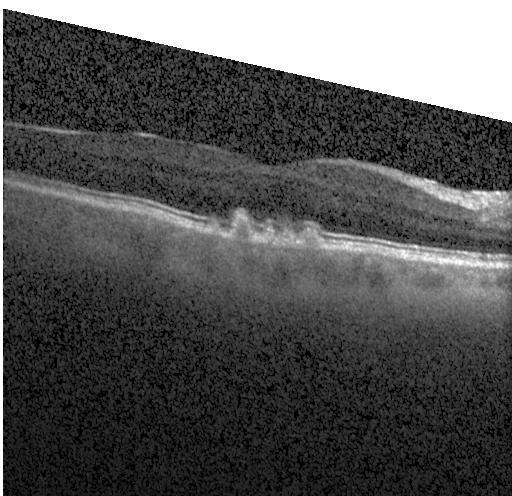

Retinal OCT B-scan. Assessment: drusen.